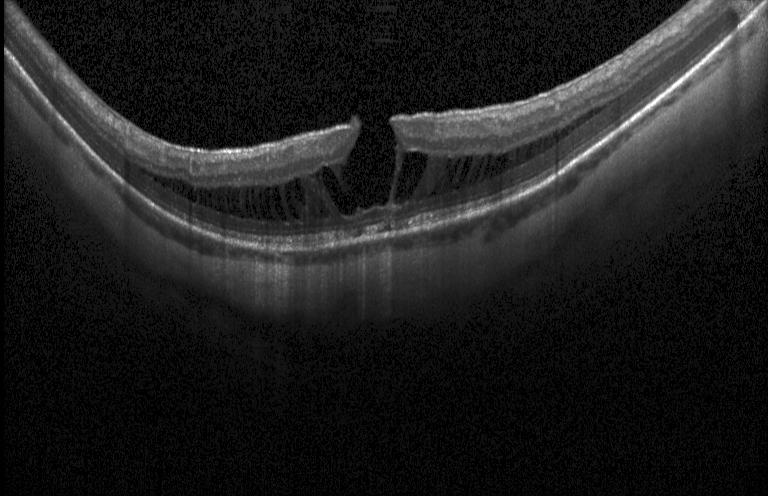 Retinal OCT B-scan. Horizontal scan through the fovea. Heidelberg Spectralis OCT system.
The scan shows diabetic macular edema (DME).